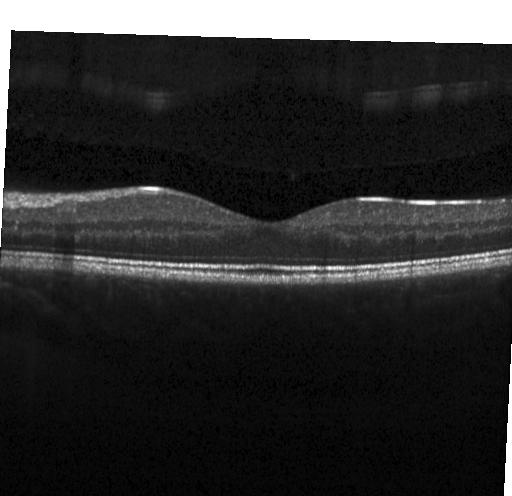 Instrument: Heidelberg Spectralis. Optical coherence tomography scan.
Dx: no choroidal neovascularization, no diabetic macular edema, and no drusen.